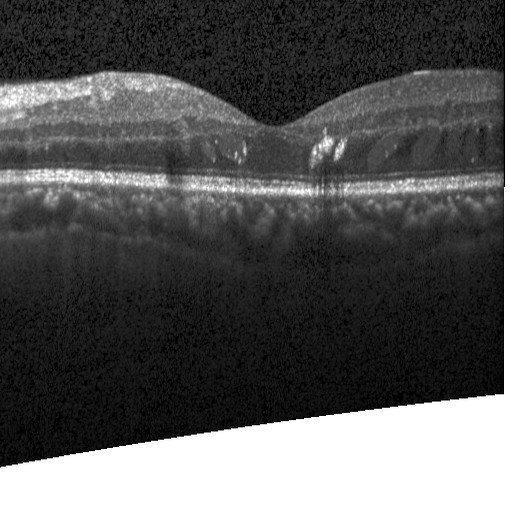 OCT finding: DME.